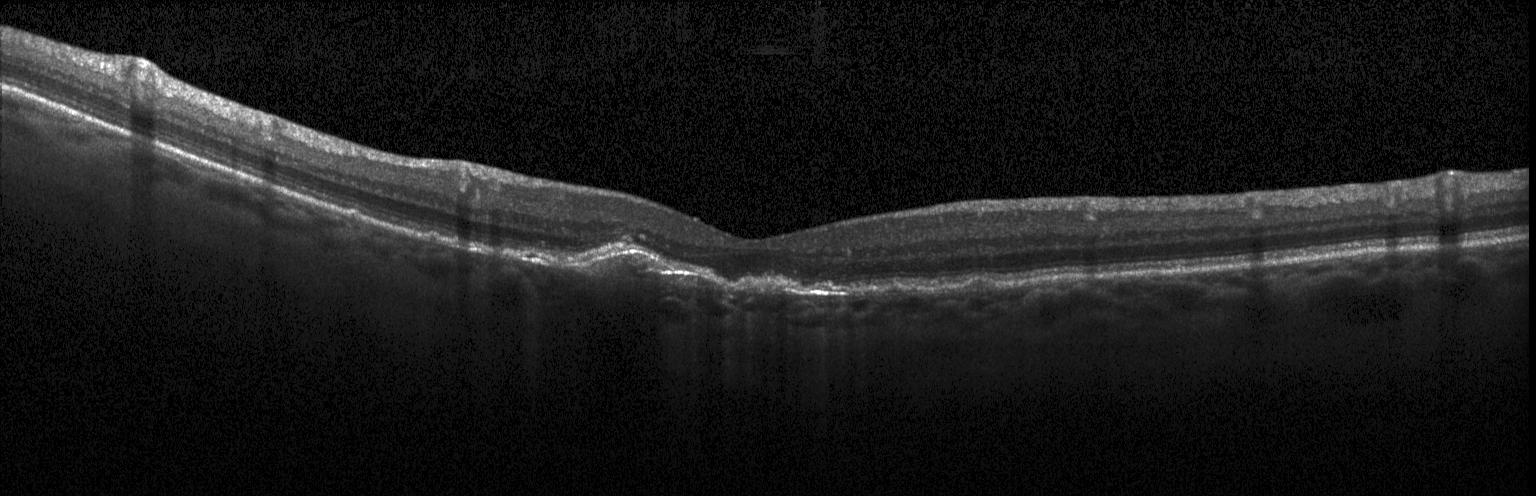
Spectral-domain optical coherence tomography. Horizontal scan through the fovea. Retinal OCT cross-section. OCT finding: a choroidal neovascular membrane.